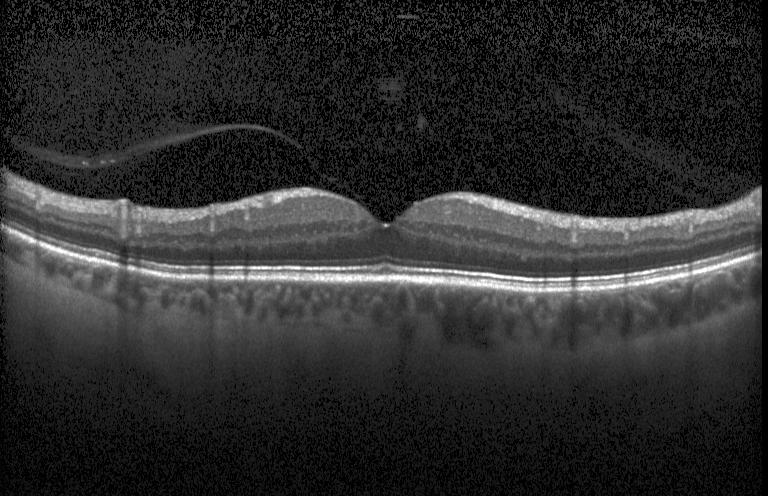 This B-scan demonstrates no choroidal neovascularization, no diabetic macular edema, and no drusen.